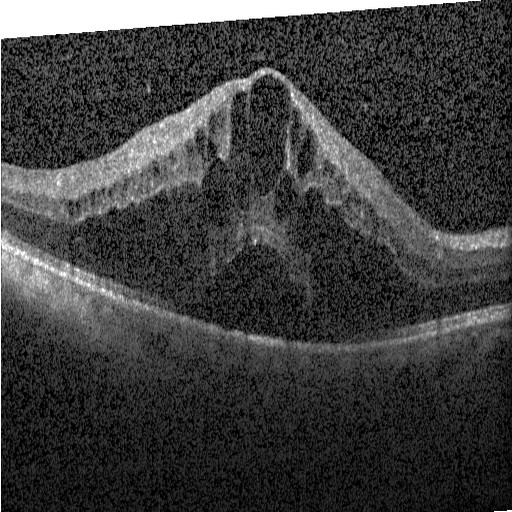 Through the macula; spectral-domain optical coherence tomography; optical coherence tomography B-scan; Heidelberg Spectralis OCT system
Assessment: diabetic macular edema.